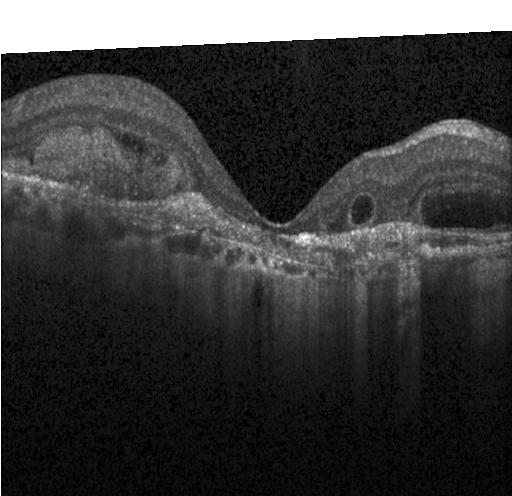
OCT B-scan showing a choroidal neovascular membrane.